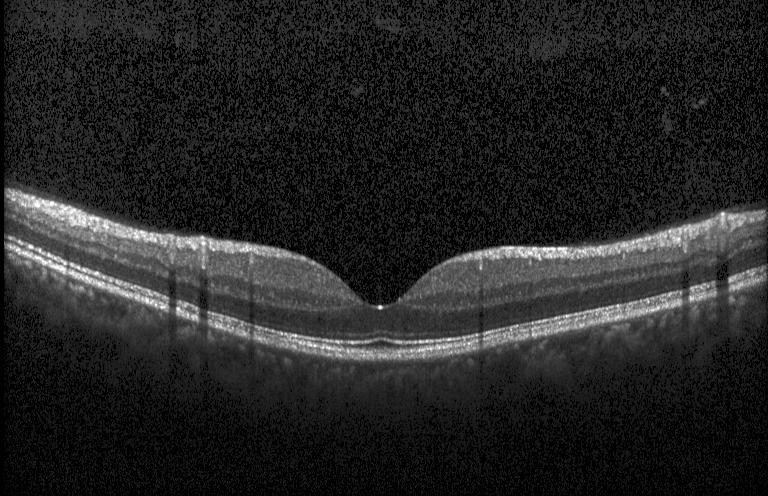 No choroidal neovascularization, diabetic macular edema, or drusen.